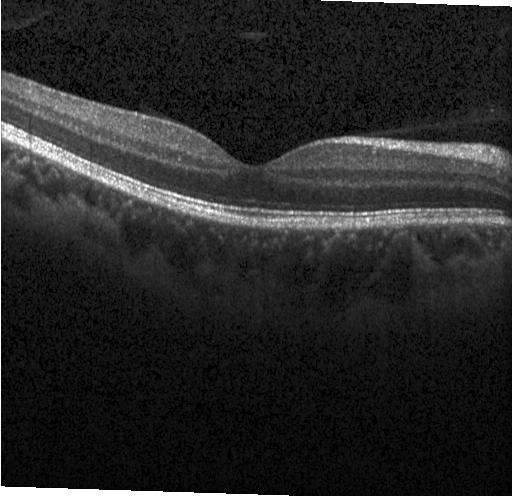
Horizontal scan through the fovea, Heidelberg Spectralis, spectral-domain optical coherence tomography, retinal OCT cross-section — No evidence of choroidal neovascularization, diabetic macular edema, or drusen.